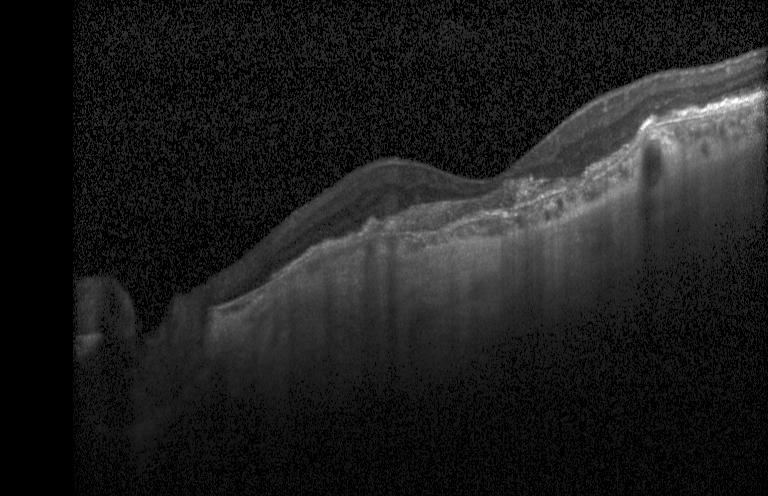

OCT scan showing choroidal neovascularization.